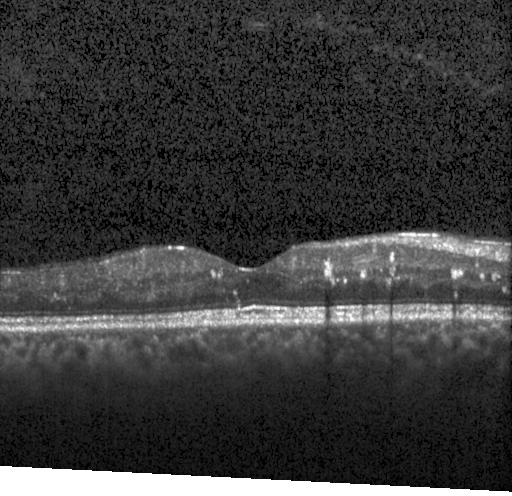 Optical coherence tomography scan
Impression: diabetic macular edema.